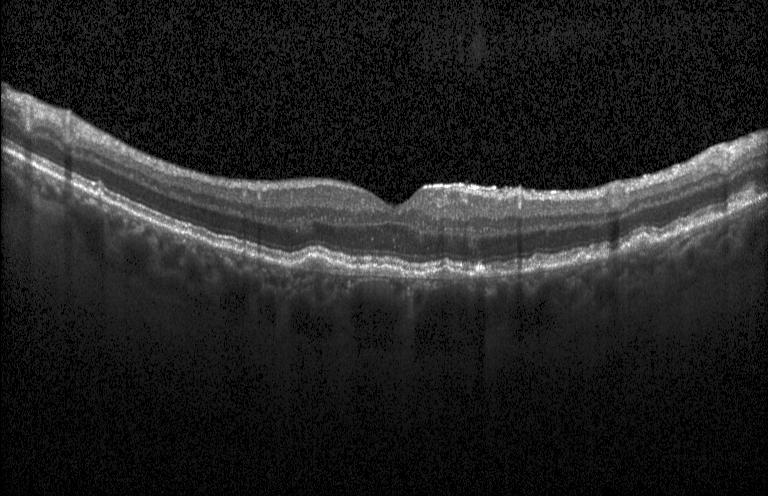 Optical coherence tomography scan — CNV.